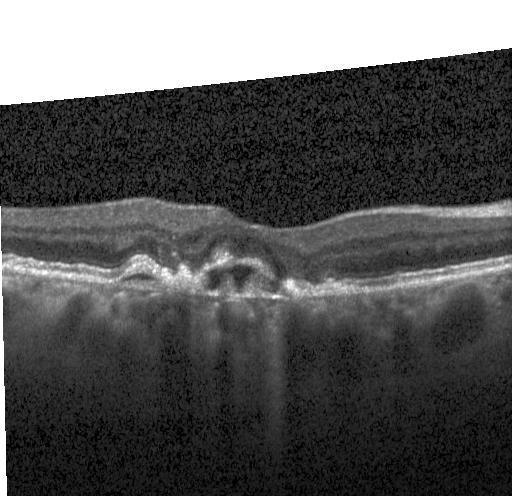 Retinal OCT cross-section
Dx: a choroidal neovascular membrane.